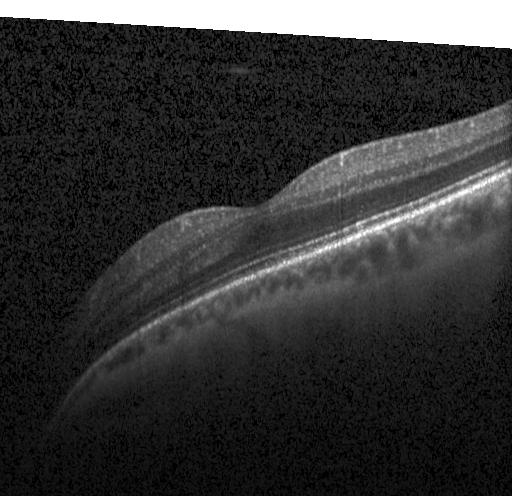
Impression: neither CNV, DME, nor drusen.